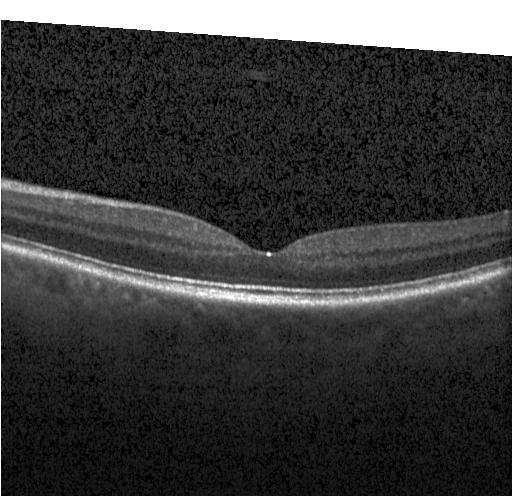 OCT finding: no choroidal neovascularization, no diabetic macular edema, and no drusen.